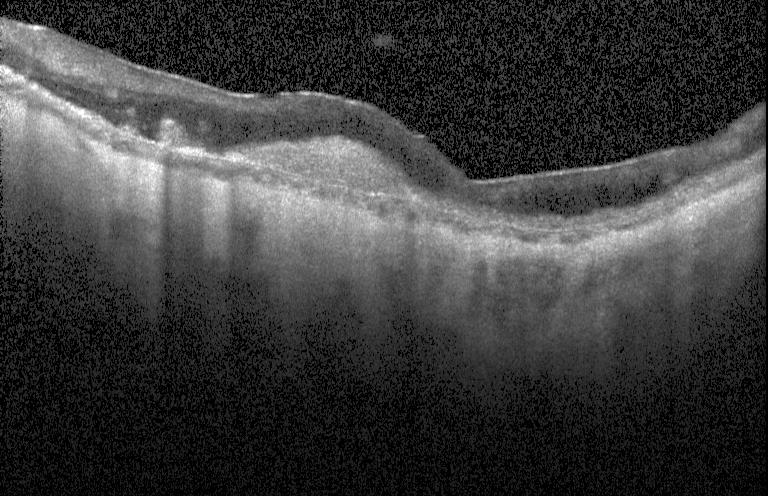
OCT B-scan. Impression: a choroidal neovascular membrane.